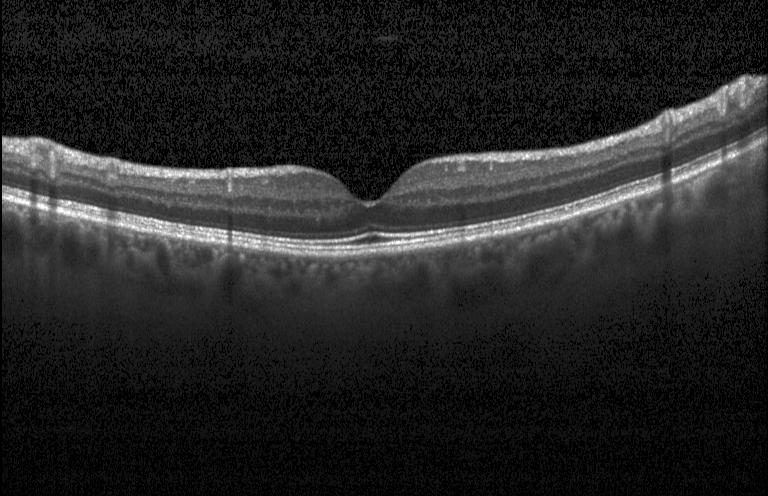 OCT line scan, spectral-domain OCT
No choroidal neovascularization, diabetic macular edema, or drusen.